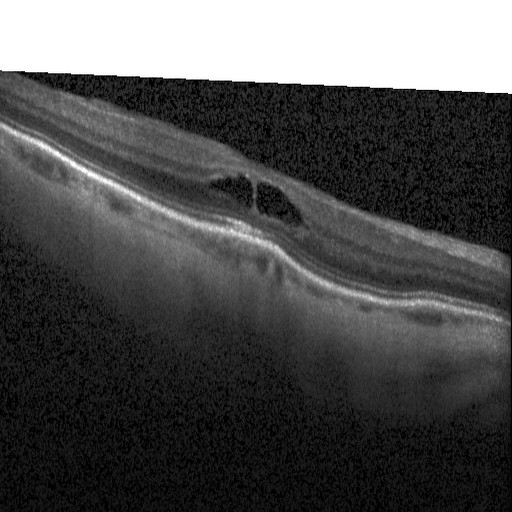
OCT scan showing DME.